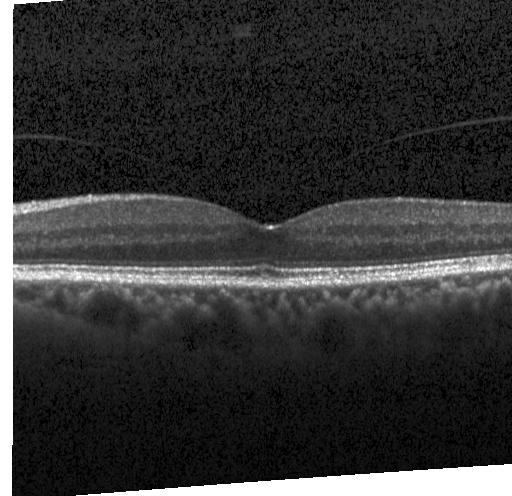 Dx: neither CNV, DME, nor drusen.